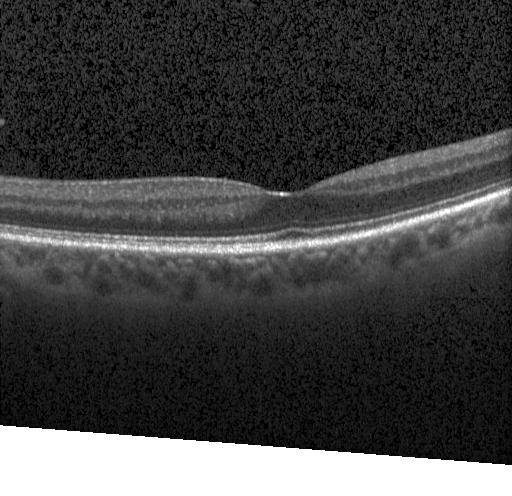
OCT finding: neither choroidal neovascularization, diabetic macular edema, nor drusen.